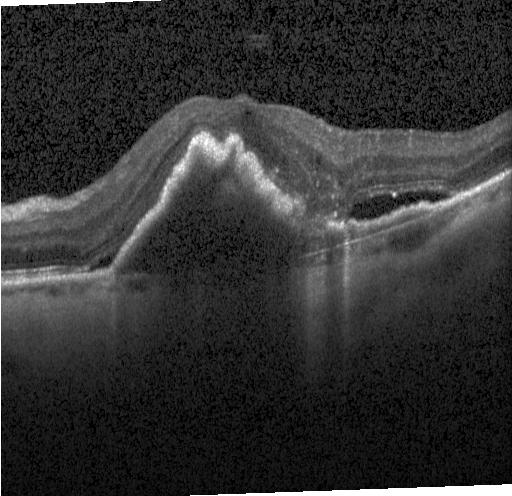

Optical coherence tomography scan, spectral-domain OCT, horizontal scan through the fovea, acquired on a Heidelberg Spectralis
This B-scan demonstrates CNV.